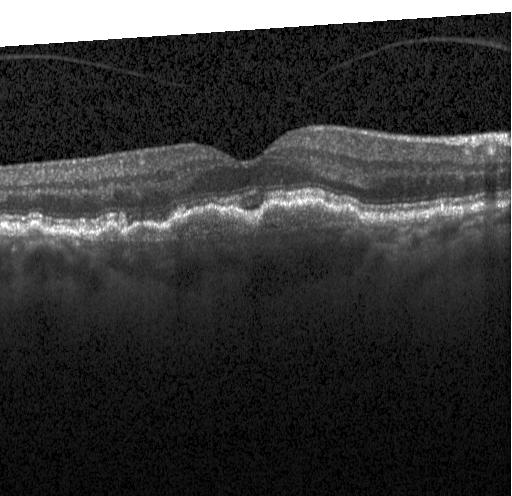
Macular scan; retinal OCT B-scan; Heidelberg Spectralis. Finding: choroidal neovascularization.